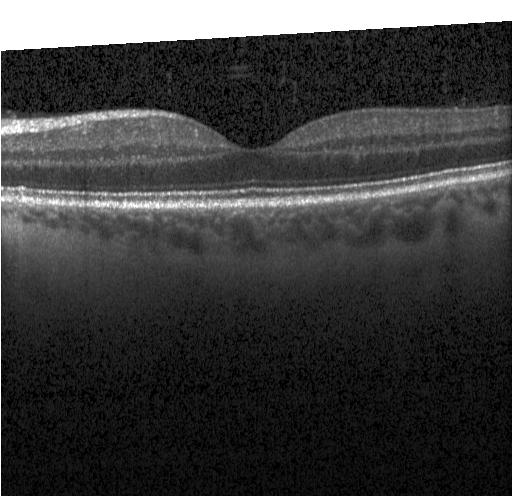

Instrument: Heidelberg Spectralis · horizontal scan through the fovea · retinal OCT B-scan · spectral-domain optical coherence tomography — Dx: neither choroidal neovascularization, diabetic macular edema, nor drusen.